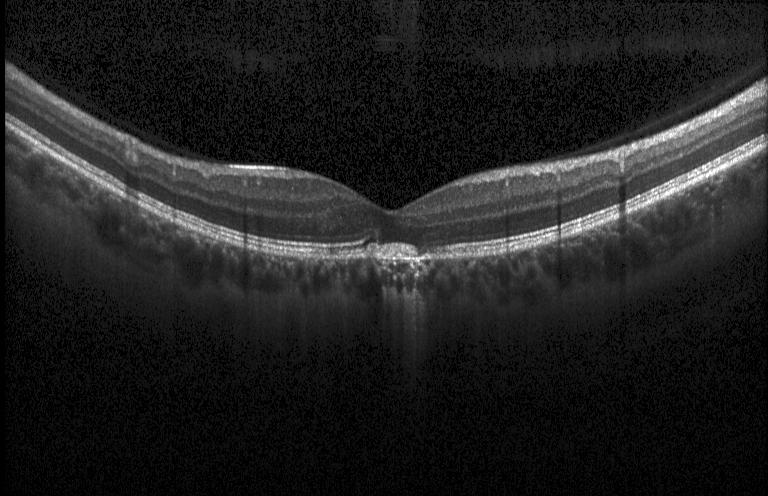 Retinal OCT cross-section showing choroidal neovascularization (CNV).